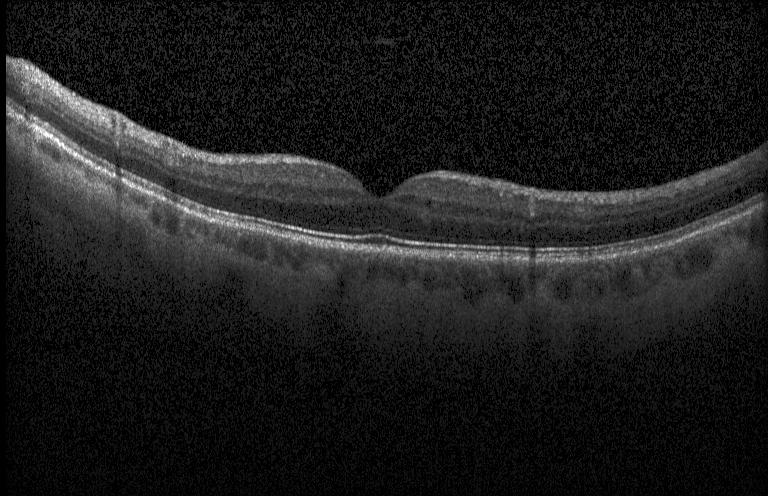

Macular scan · spectral-domain optical coherence tomography · optical coherence tomography B-scan. Macular OCT: no CNV, DME, or drusen.